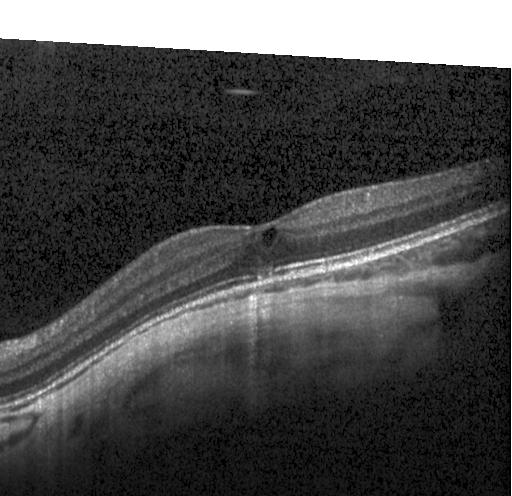
Impression: DME.